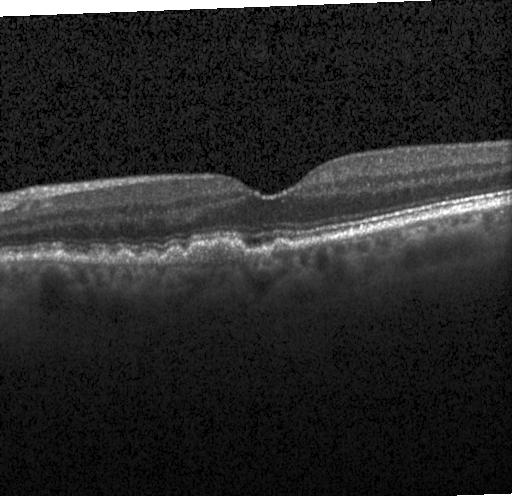
Macular OCT demonstrating multiple drusen.